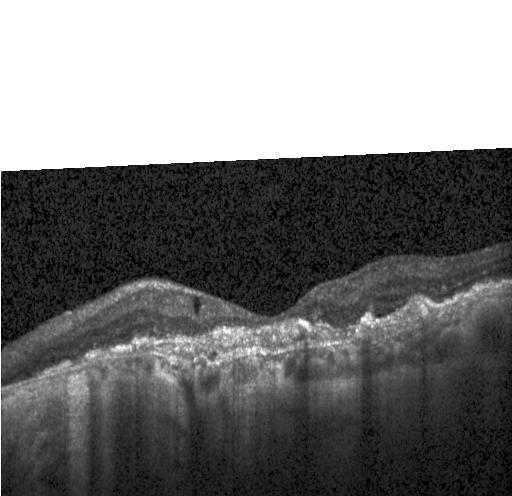
Retinal OCT cross-section. Heidelberg Spectralis
Diagnosis: choroidal neovascularization.